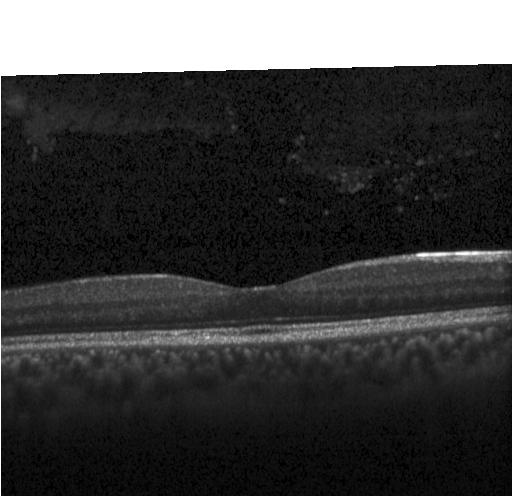 Diagnosis: neither CNV, DME, nor drusen.